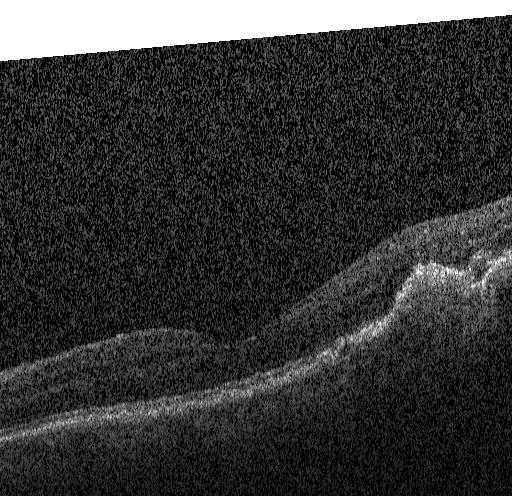
Macular scan; spectral-domain optical coherence tomography; Heidelberg Spectralis OCT system; retinal OCT cross-section.
Assessment: a choroidal neovascular membrane.